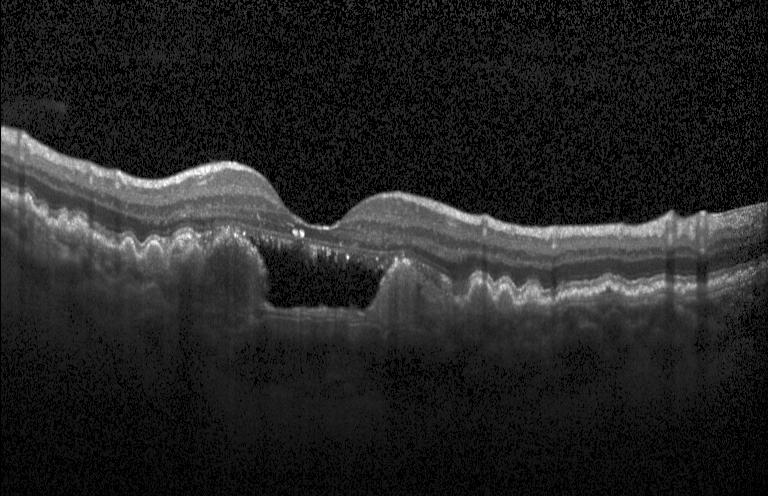
Finding: choroidal neovascularization (CNV).